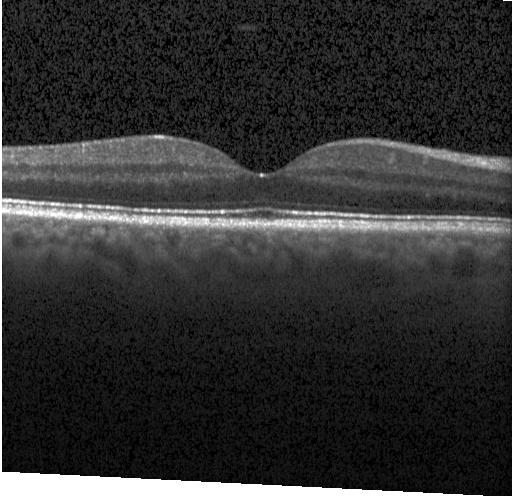
Assessment: neither choroidal neovascularization, diabetic macular edema, nor drusen.